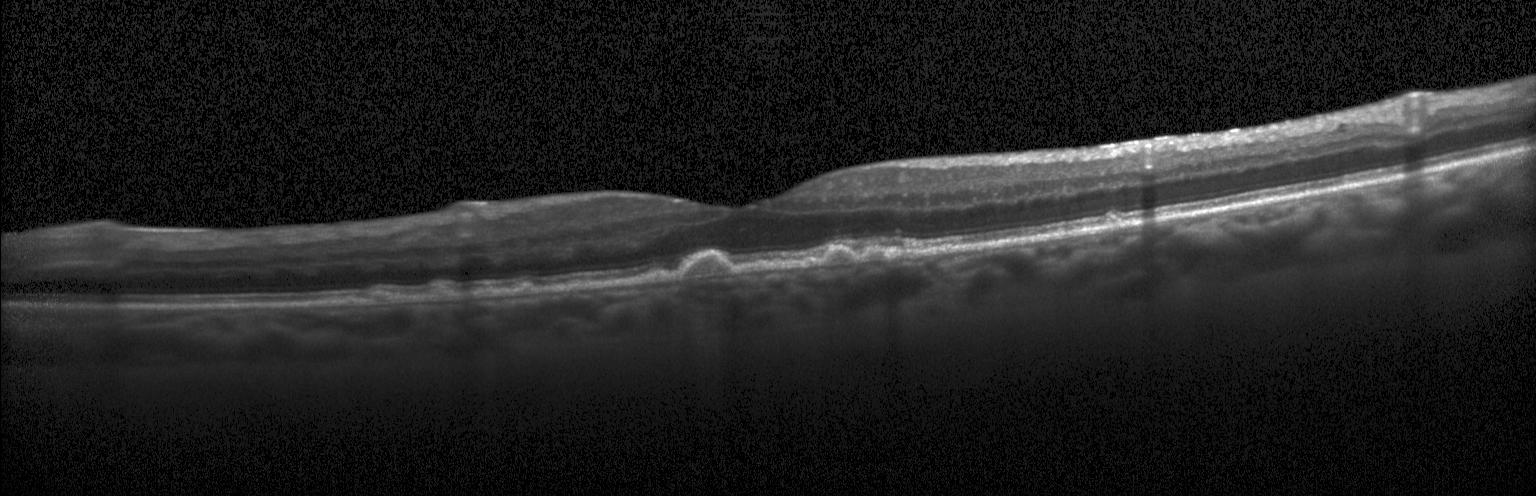

OCT B-scan showing multiple drusen.